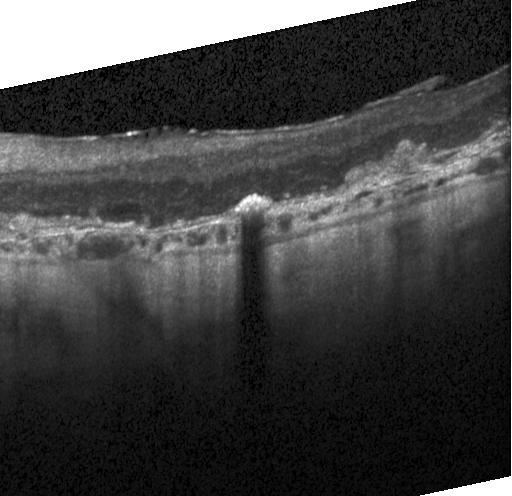 Spectral-domain optical coherence tomography, Heidelberg Spectralis, optical coherence tomography scan
This B-scan demonstrates choroidal neovascularization.